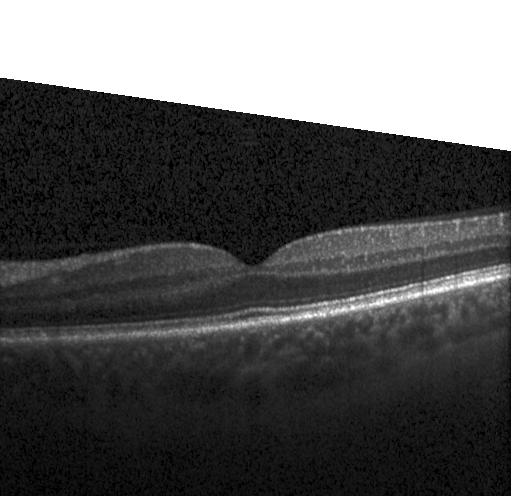
Instrument: Heidelberg Spectralis; spectral-domain optical coherence tomography; retinal OCT B-scan; centered on the fovea — Dx: no choroidal neovascularization, diabetic macular edema, or drusen.